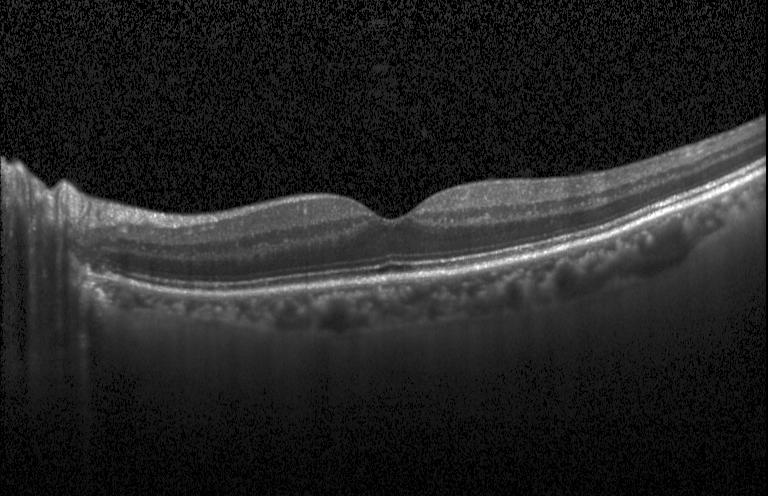
Retinal OCT cross-section · spectral-domain OCT · macular scan — Macular OCT: no evidence of choroidal neovascularization, diabetic macular edema, or drusen.